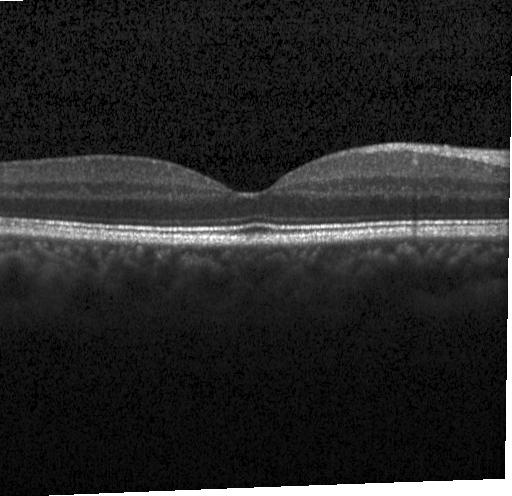 OCT B-scan. Macular scan. Heidelberg Spectralis. Spectral-domain optical coherence tomography. This B-scan demonstrates no CNV, no DME, and no drusen.